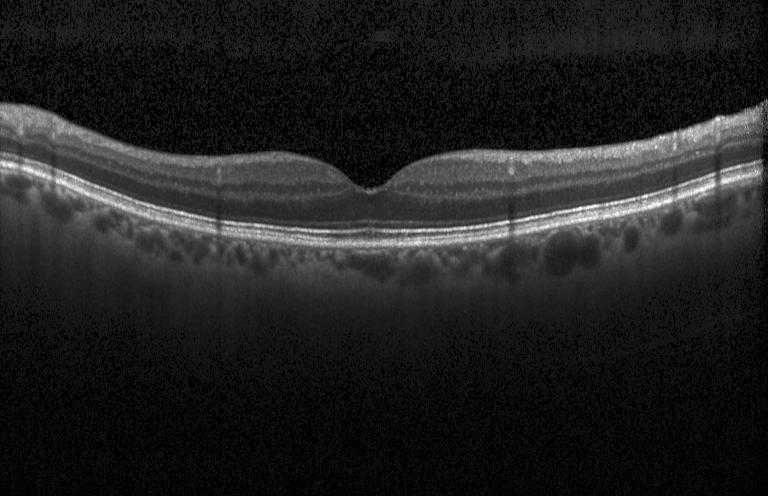
Impression: no evidence of choroidal neovascularization, diabetic macular edema, or drusen.